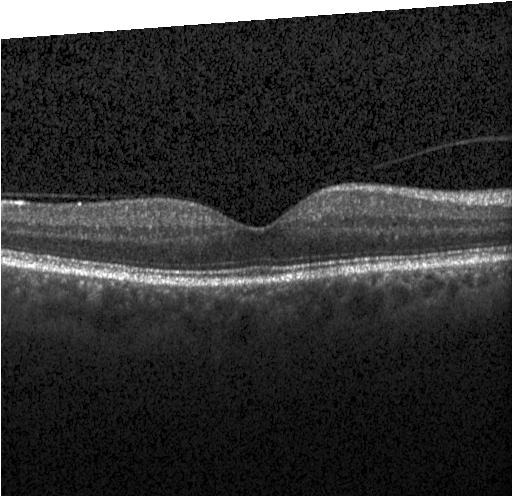
Spectral-domain optical coherence tomography. Optical coherence tomography B-scan
Impression: neither choroidal neovascularization, diabetic macular edema, nor drusen.